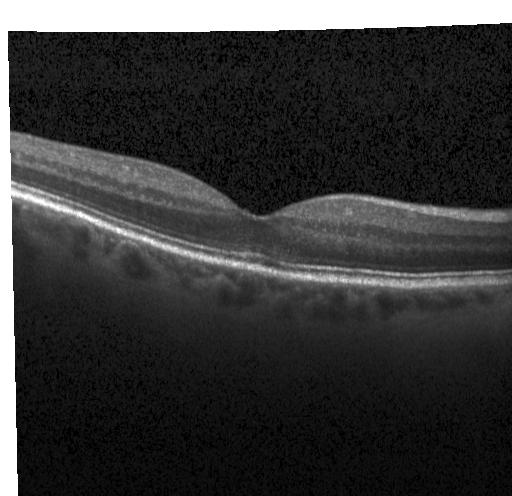 OCT line scan.
OCT finding: no CNV, no DME, and no drusen.